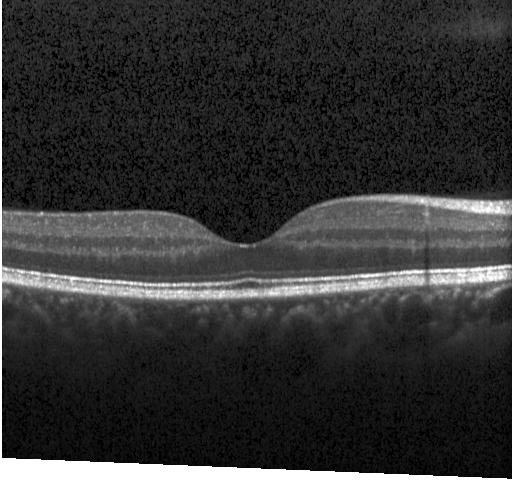 SD-OCT; horizontal scan through the fovea; Heidelberg Spectralis OCT system; optical coherence tomography B-scan. Diagnosis: no choroidal neovascularization, diabetic macular edema, or drusen.